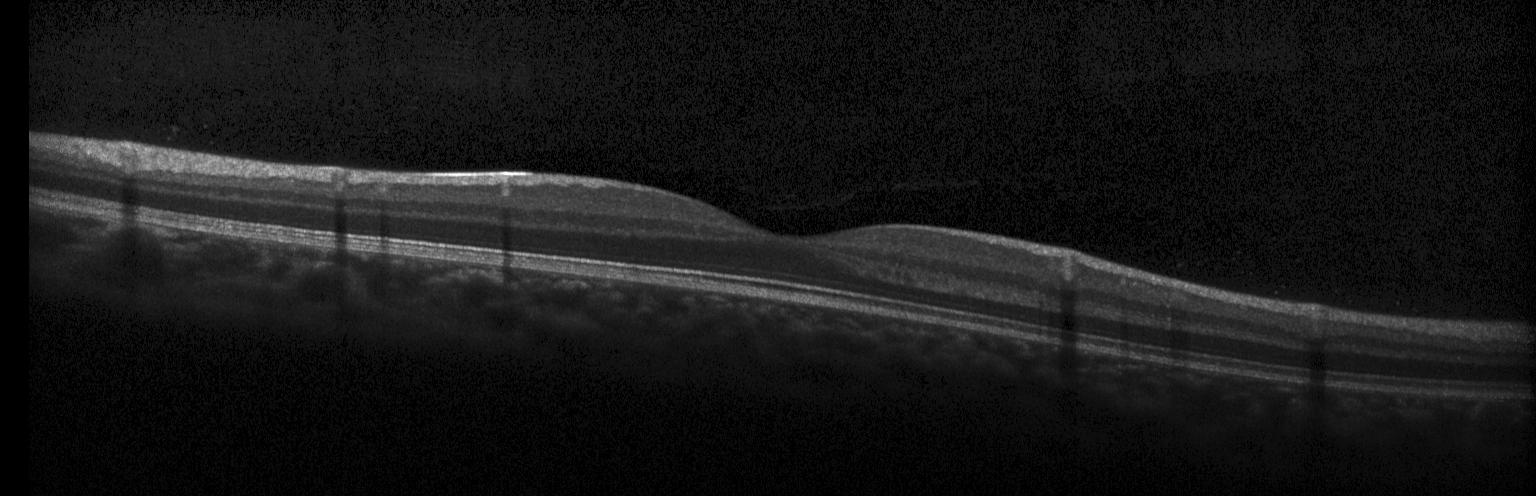

Assessment: no evidence of CNV, DME, or drusen.